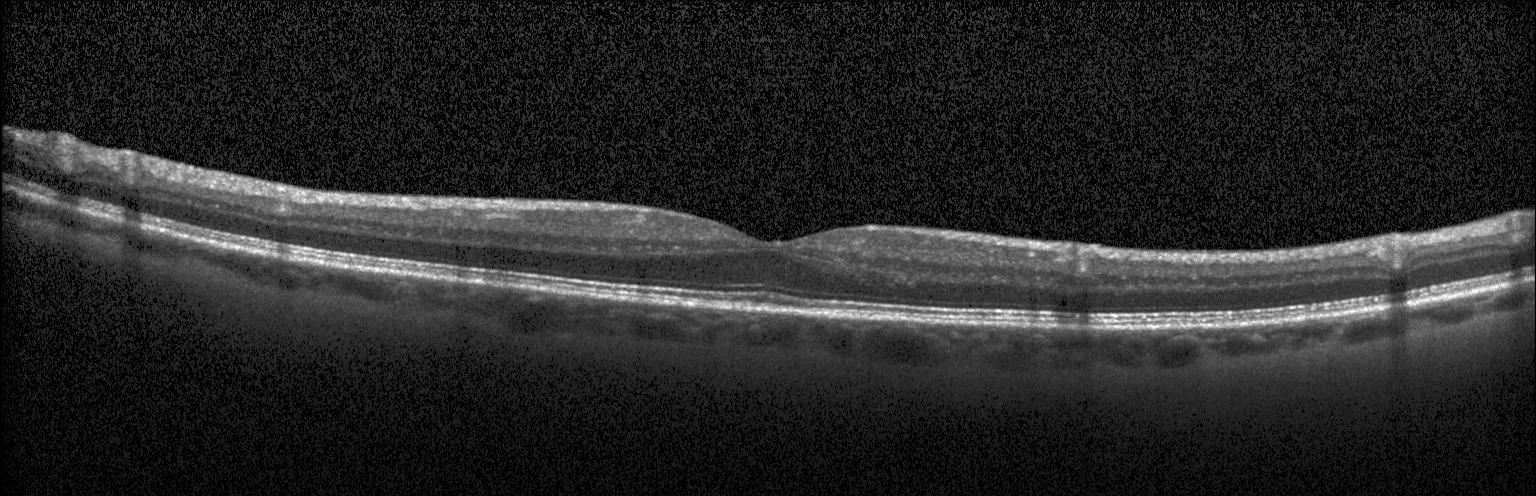 Retinal OCT cross-section, spectral-domain OCT, through the macula, instrument: Heidelberg Spectralis — Macular OCT: no choroidal neovascularization, no diabetic macular edema, and no drusen.